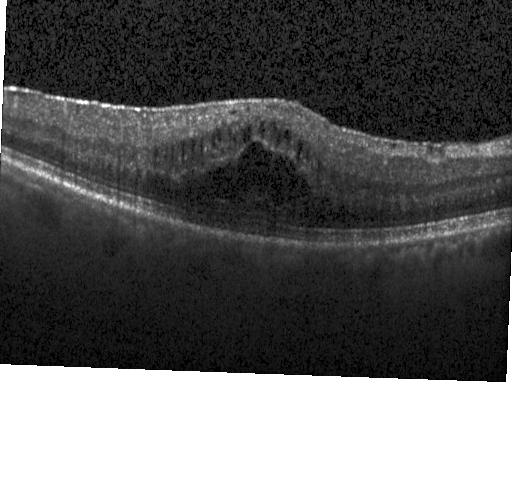
Centered on the fovea · optical coherence tomography B-scan.
Impression: DME.